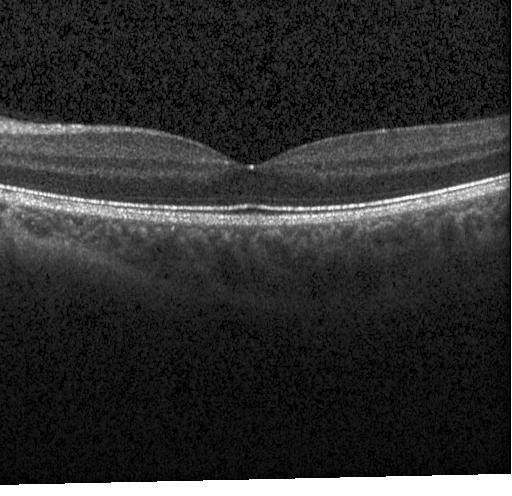 Diagnosis: neither choroidal neovascularization, diabetic macular edema, nor drusen.